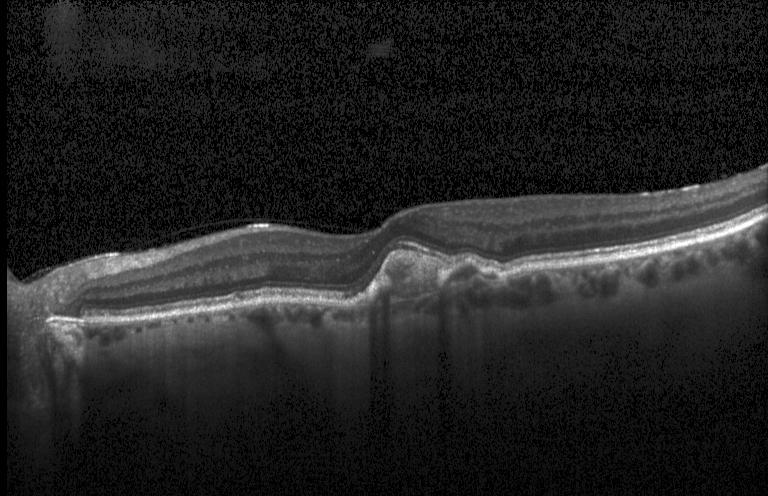

OCT line scan
Dx: CNV.